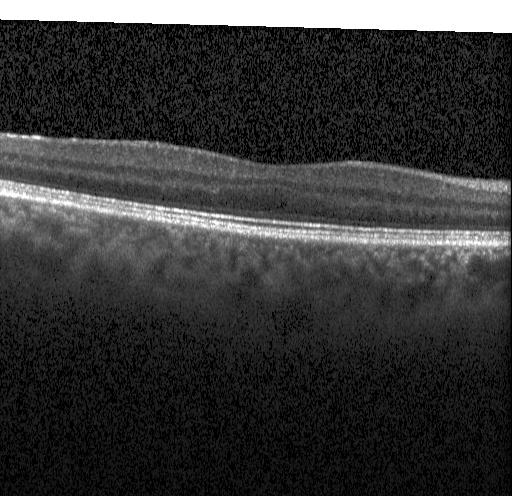
Finding: neither choroidal neovascularization, diabetic macular edema, nor drusen.